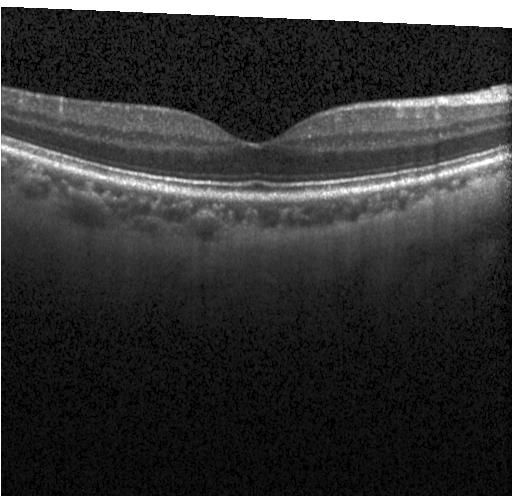
Instrument: Heidelberg Spectralis · optical coherence tomography scan · SD-OCT.
Diagnosis: no evidence of choroidal neovascularization, diabetic macular edema, or drusen.